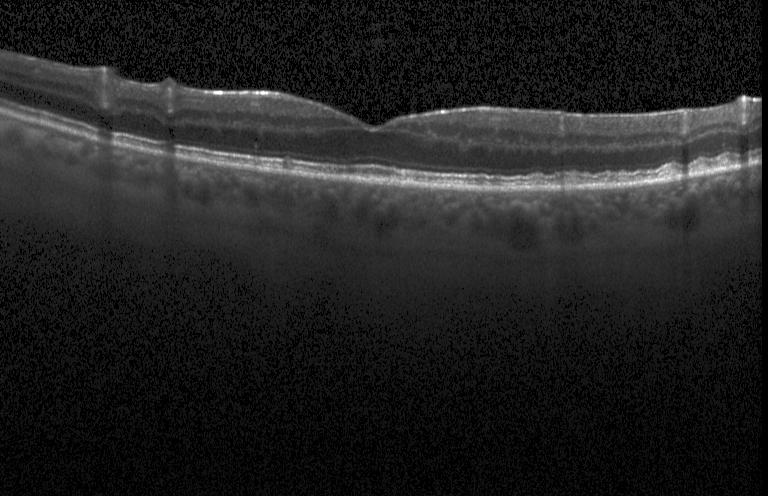

OCT B-scan showing no evidence of CNV, DME, or drusen.